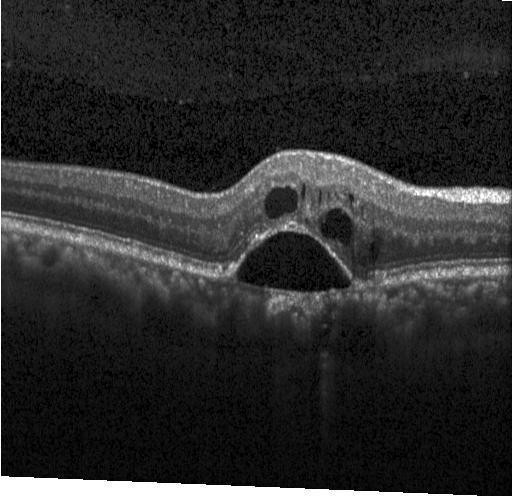
OCT line scan
Diagnosis: a choroidal neovascular membrane.